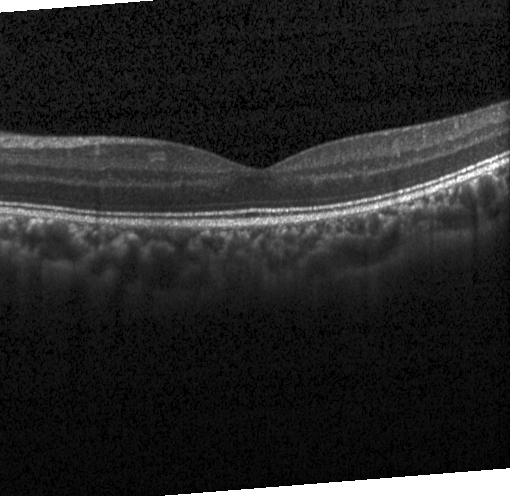

Retinal OCT cross-section — Diagnosis: no evidence of CNV, DME, or drusen.